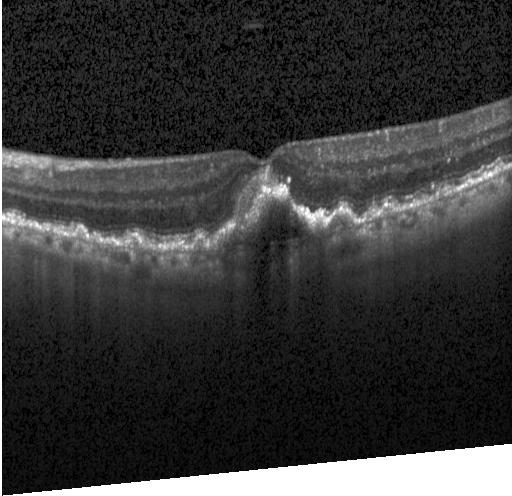 Impression: a choroidal neovascular membrane.